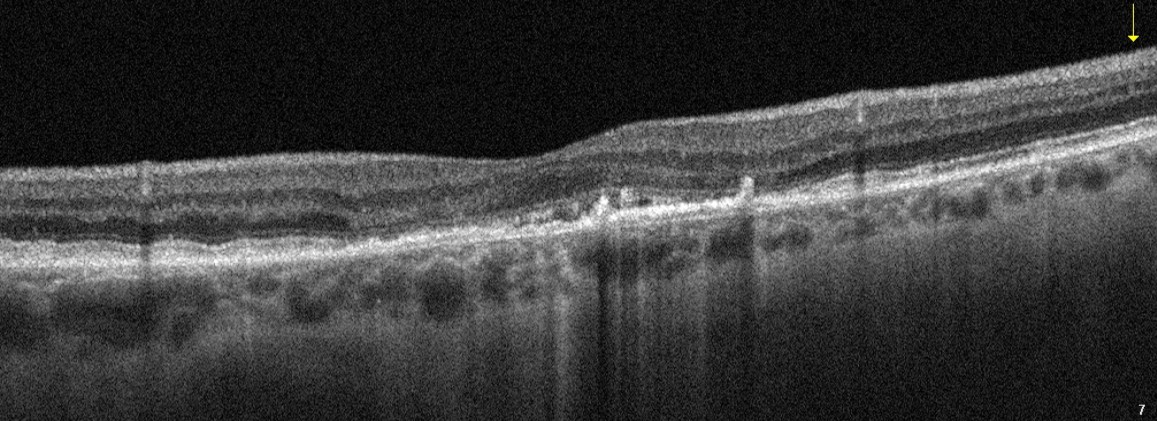
Optical coherence tomography scan. Impression: AMD.